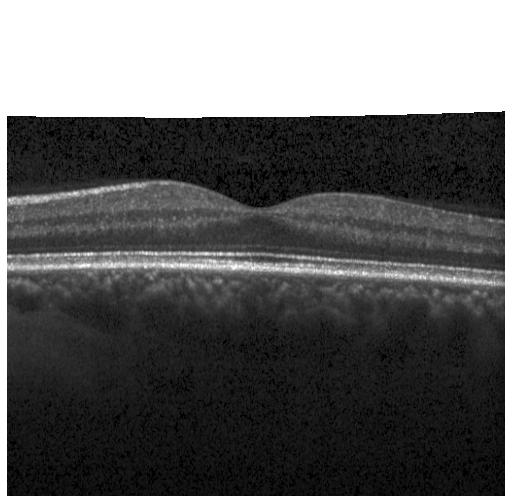 Macular OCT demonstrating no evidence of choroidal neovascularization, diabetic macular edema, or drusen.